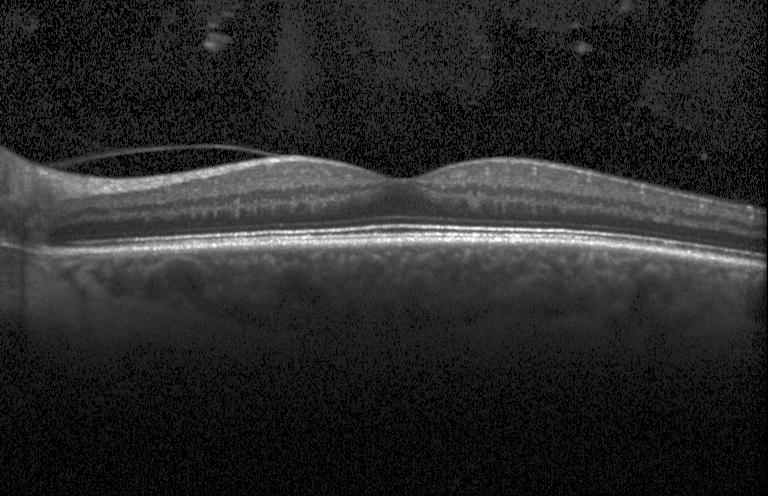

Through the macula; instrument: Heidelberg Spectralis; spectral-domain optical coherence tomography; retinal OCT cross-section. Finding: neither choroidal neovascularization, diabetic macular edema, nor drusen.